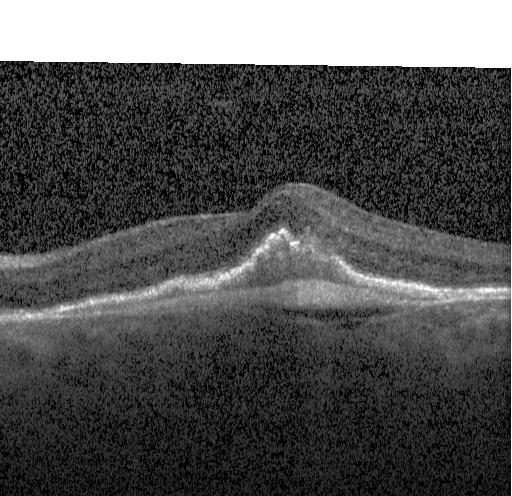

Instrument: Heidelberg Spectralis, fovea-centered, SD-OCT, optical coherence tomography B-scan — Dx: a choroidal neovascular membrane.